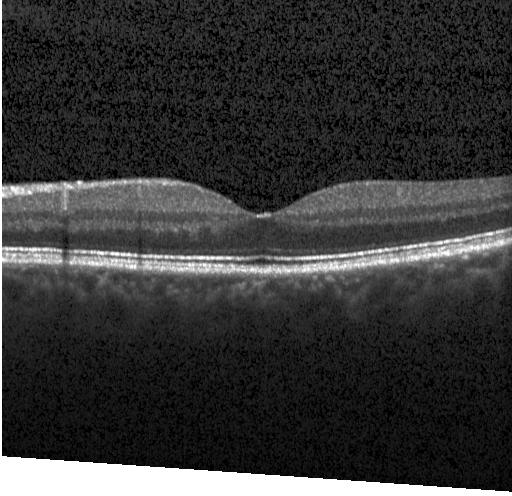
OCT scan showing no CNV, no DME, and no drusen.